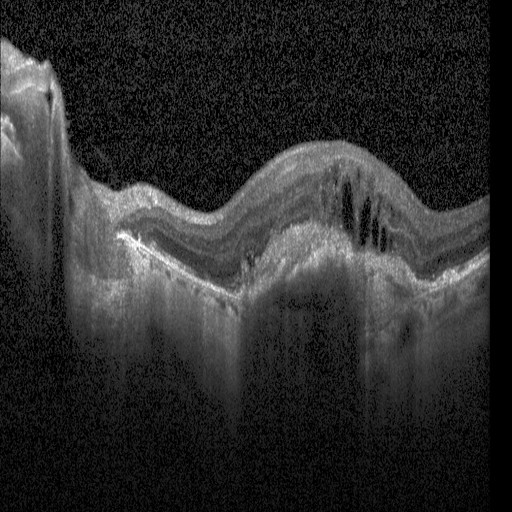

OCT line scan, Heidelberg Spectralis OCT system, horizontal scan through the fovea — Assessment: diabetic macular edema (DME).